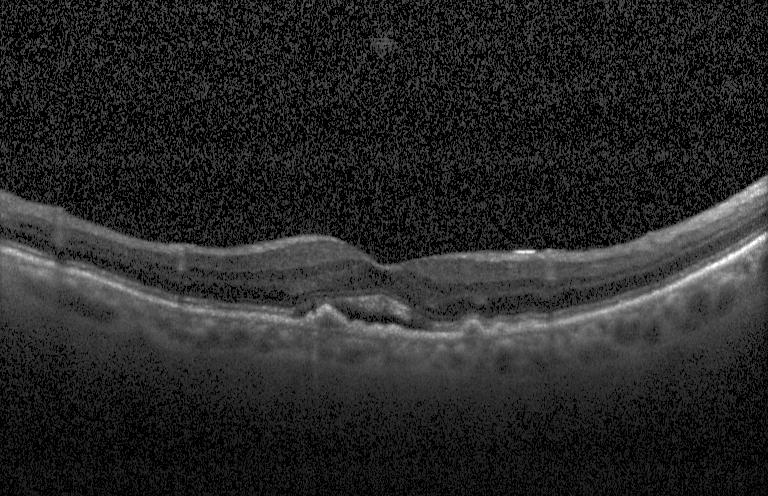

Instrument: Heidelberg Spectralis, retinal OCT B-scan — Diagnosis: choroidal neovascularization.